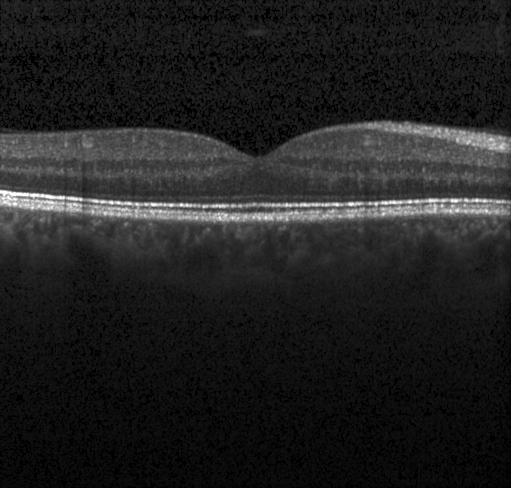 SD-OCT · optical coherence tomography scan. Assessment: neither choroidal neovascularization, diabetic macular edema, nor drusen.